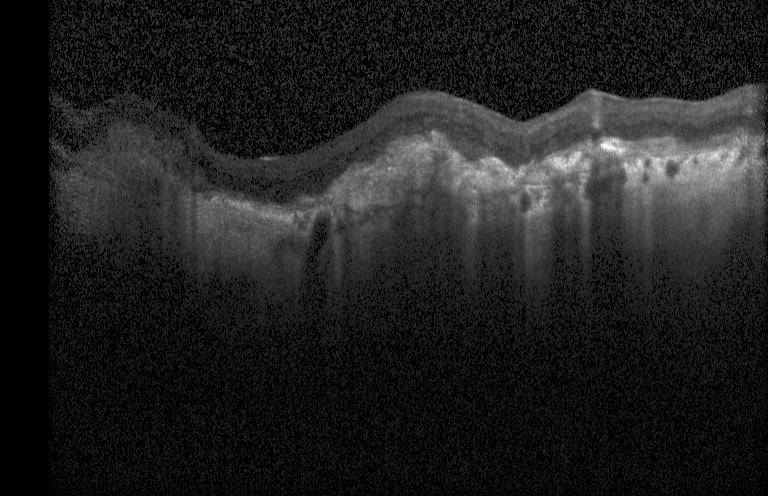

Finding: a choroidal neovascular membrane.